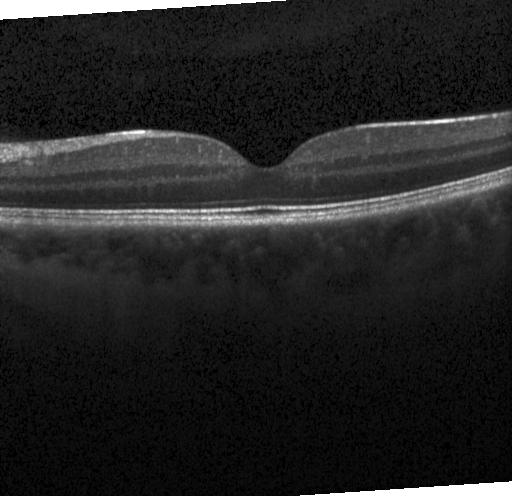
Acquired on a Heidelberg Spectralis. OCT B-scan. Macular scan.
OCT finding: no choroidal neovascularization, diabetic macular edema, or drusen.